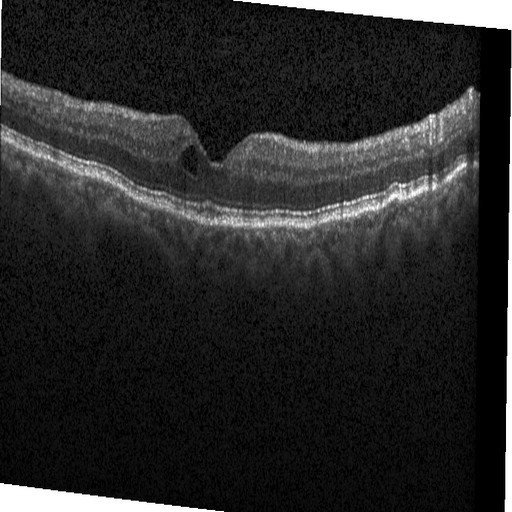 Impression: diabetic macular edema (DME).